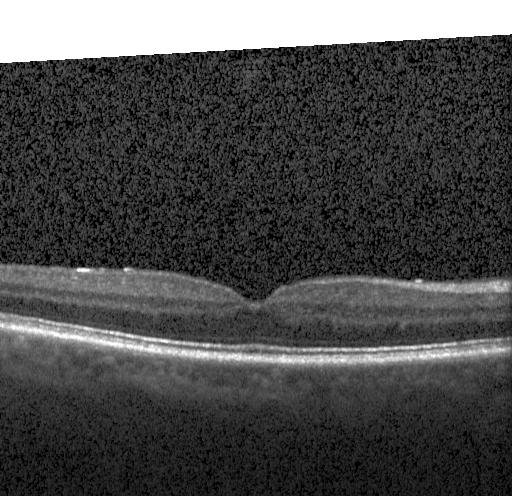 OCT B-scan. Impression: no choroidal neovascularization, no diabetic macular edema, and no drusen.